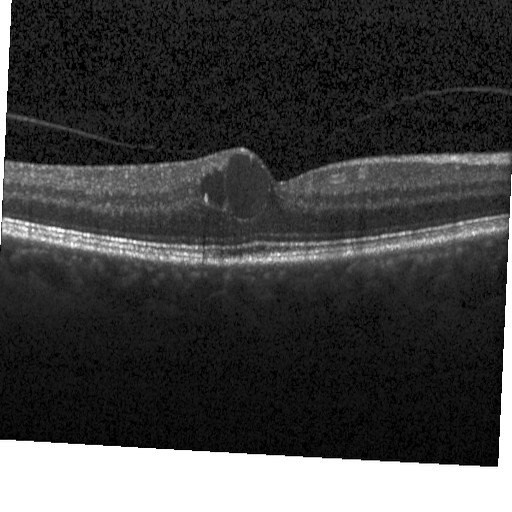

Dx: diabetic macular edema (DME).